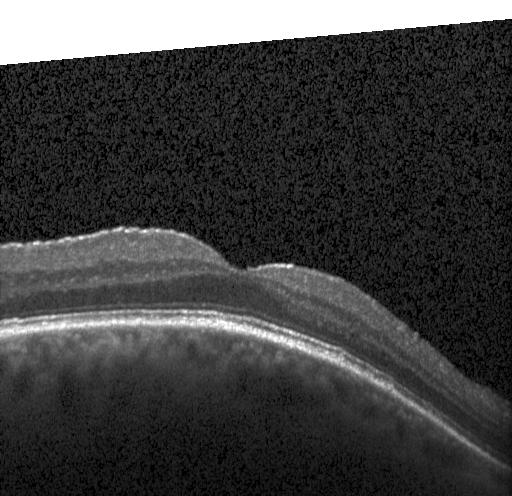 This B-scan demonstrates neither choroidal neovascularization, diabetic macular edema, nor drusen.